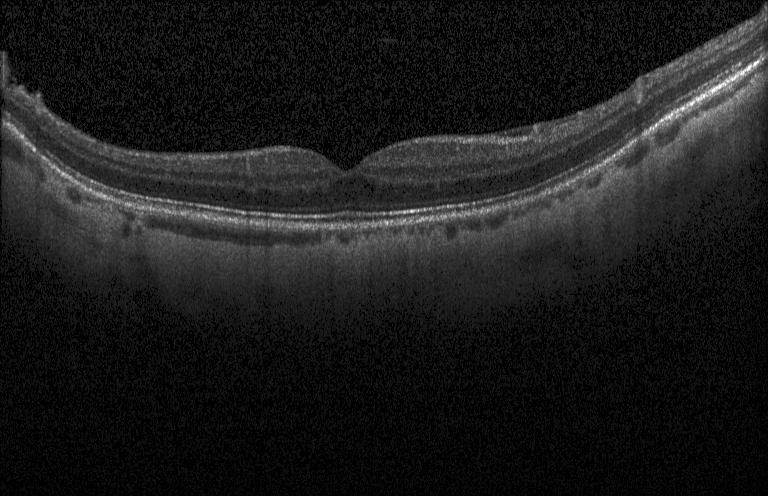 Optical coherence tomography scan. Heidelberg Spectralis. Centered on the fovea. Assessment: no evidence of choroidal neovascularization, diabetic macular edema, or drusen.